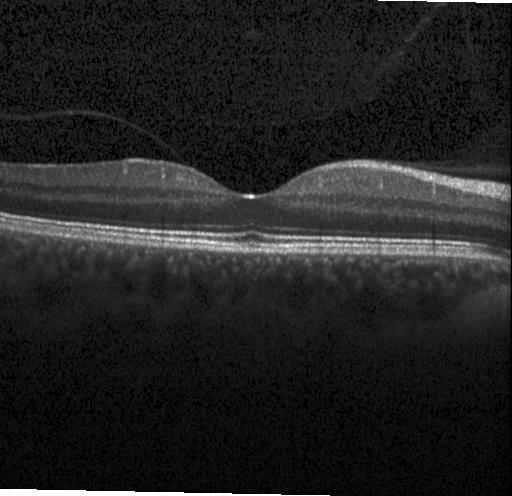
Retinal OCT B-scan
Diagnosis: no evidence of CNV, DME, or drusen.